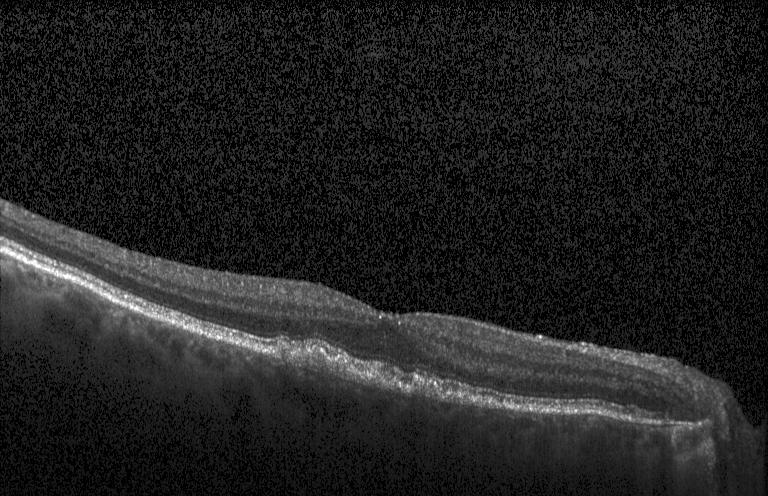
This B-scan demonstrates drusen.